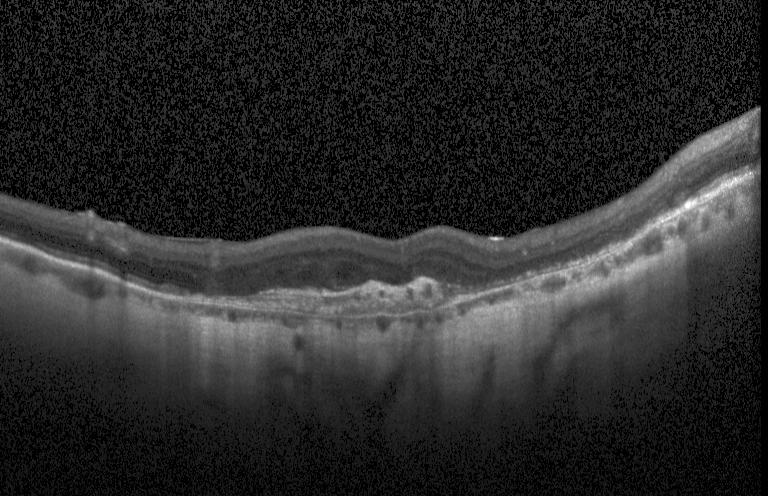
Impression: a choroidal neovascular membrane.